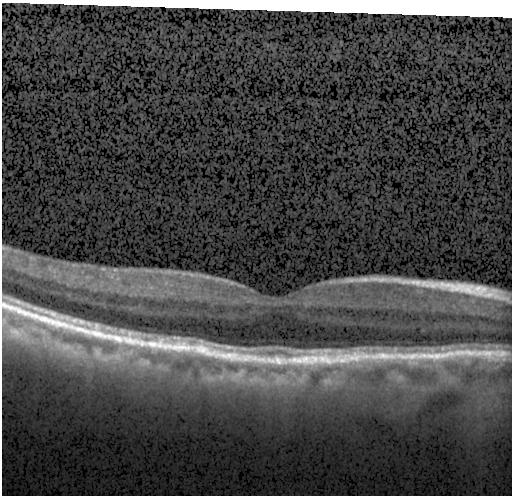
Diagnosis: neither CNV, DME, nor drusen.